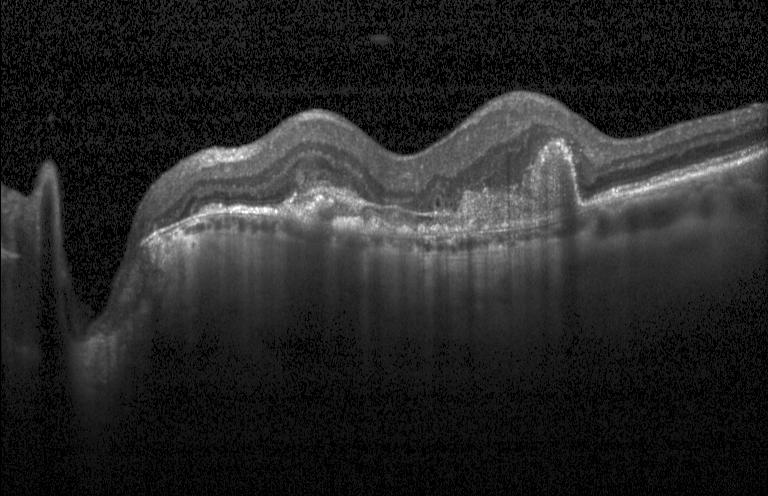

SD-OCT, instrument: Heidelberg Spectralis, retinal OCT cross-section. The scan shows choroidal neovascularization (CNV).